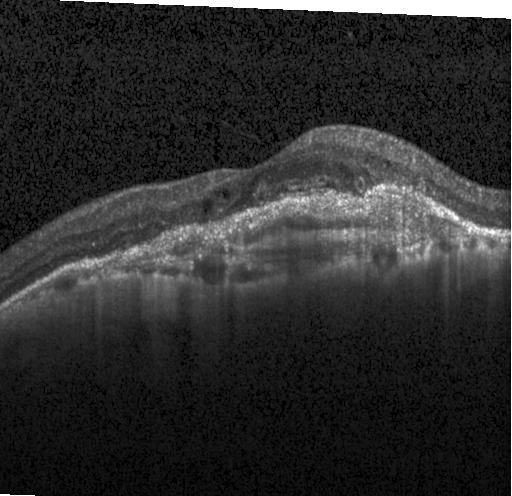
Optical coherence tomography B-scan. Diagnosis: a choroidal neovascular membrane.